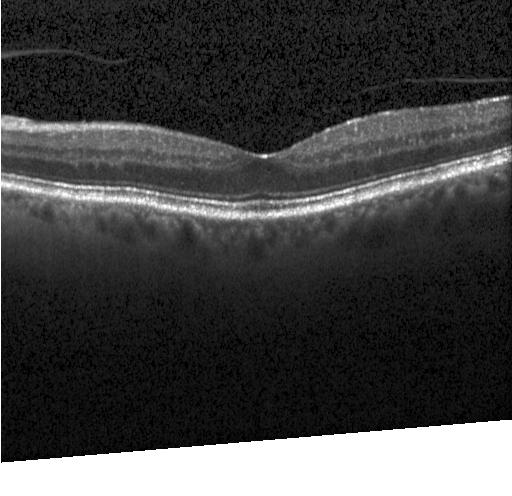
Optical coherence tomography B-scan.
Impression: no evidence of choroidal neovascularization, diabetic macular edema, or drusen.